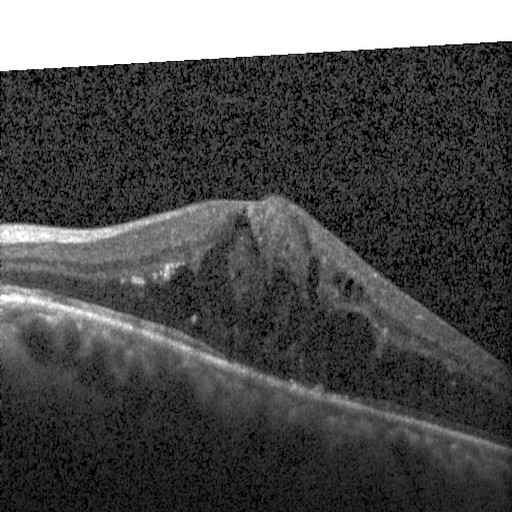 Diabetic macular edema (DME).